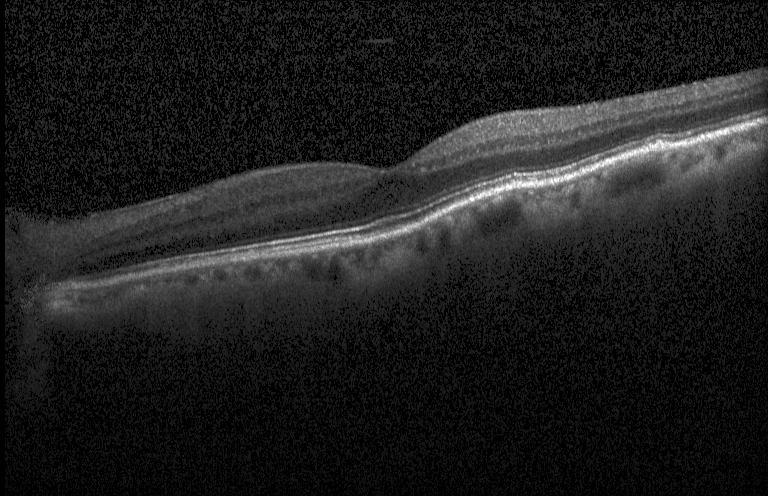
Diagnosis: neither CNV, DME, nor drusen.